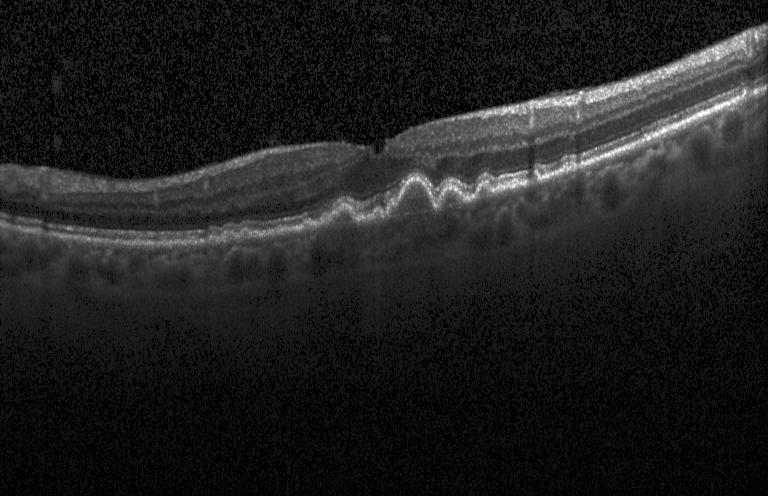 SD-OCT, through the macula, optical coherence tomography B-scan. Impression: drusen.